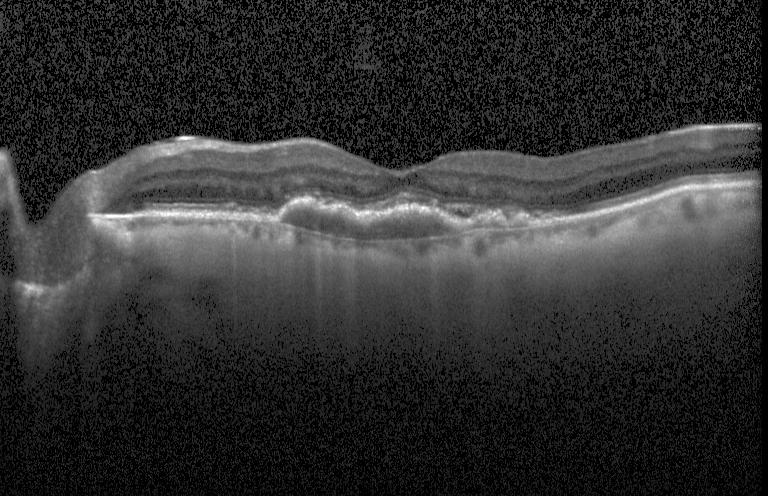
OCT B-scan.
OCT finding: CNV.